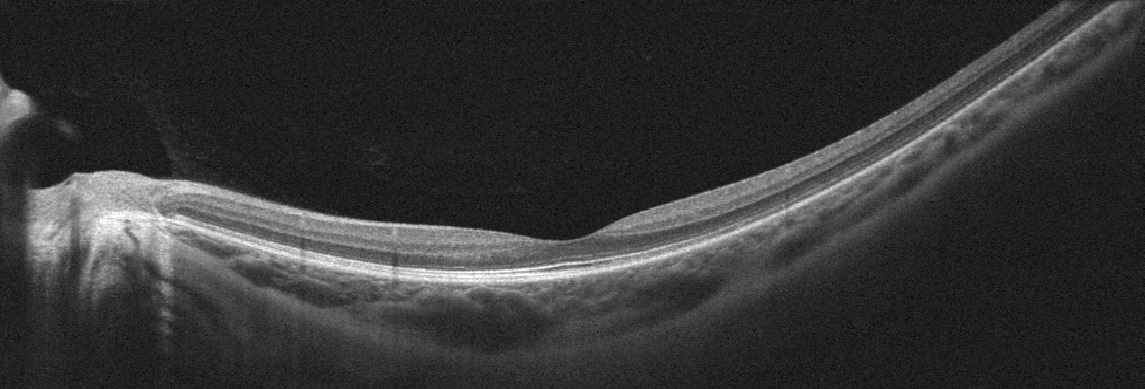

Optical coherence tomography scan — Diagnosis: no evidence of AMD, DME, ERM, RAO, RVO, or VID.